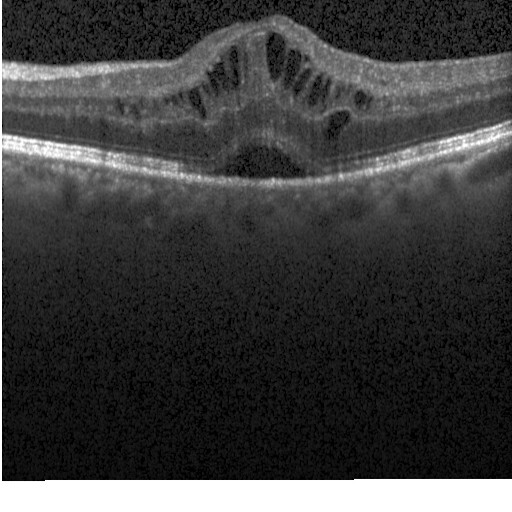

SD-OCT. Macular scan. OCT B-scan
The scan shows DME.